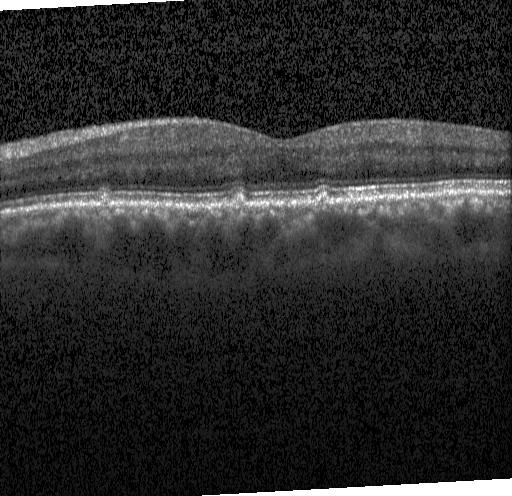 OCT B-scan showing drusen.